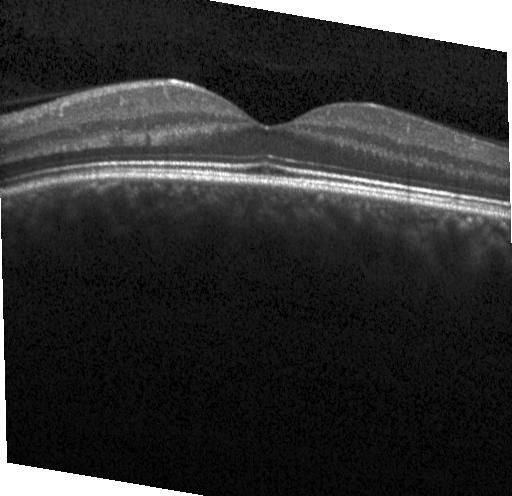 SD-OCT · optical coherence tomography scan · macular scan.
Macular OCT: no choroidal neovascularization, no diabetic macular edema, and no drusen.